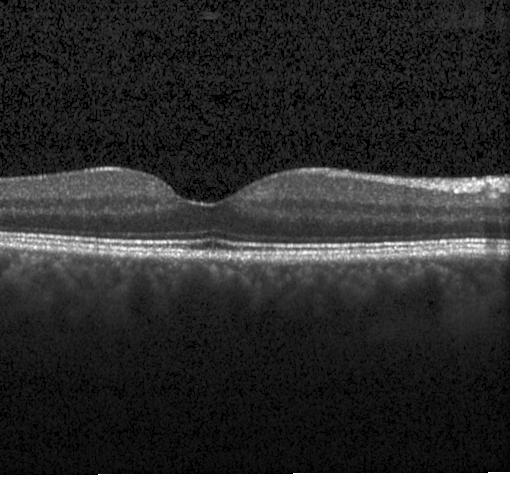

Macular OCT demonstrating no CNV, DME, or drusen.